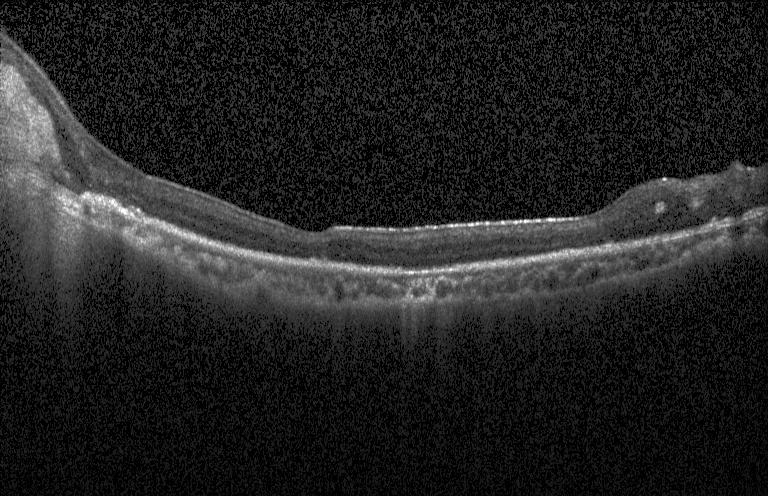

Diagnosis: CNV.